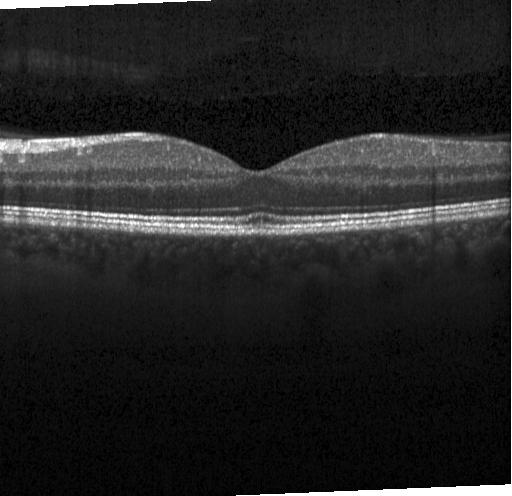 Optical coherence tomography B-scan. This B-scan demonstrates neither choroidal neovascularization, diabetic macular edema, nor drusen.